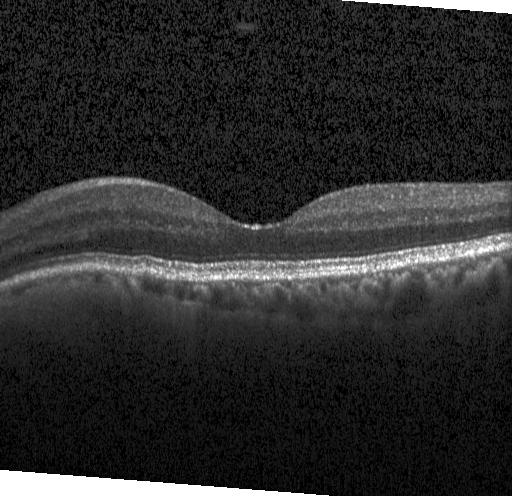 Neither CNV, DME, nor drusen.